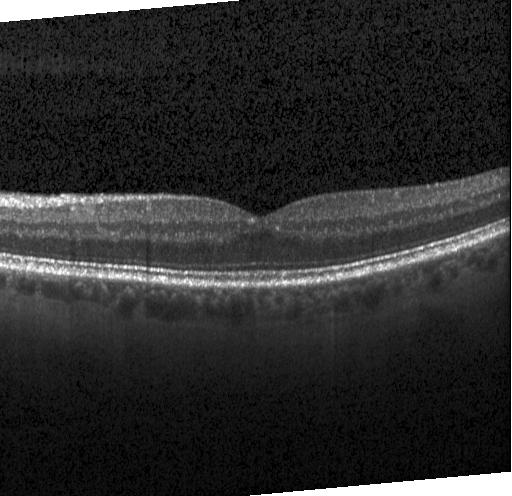
Spectral-domain optical coherence tomography · centered on the fovea · acquired on a Heidelberg Spectralis · optical coherence tomography B-scan. No CNV, DME, or drusen.